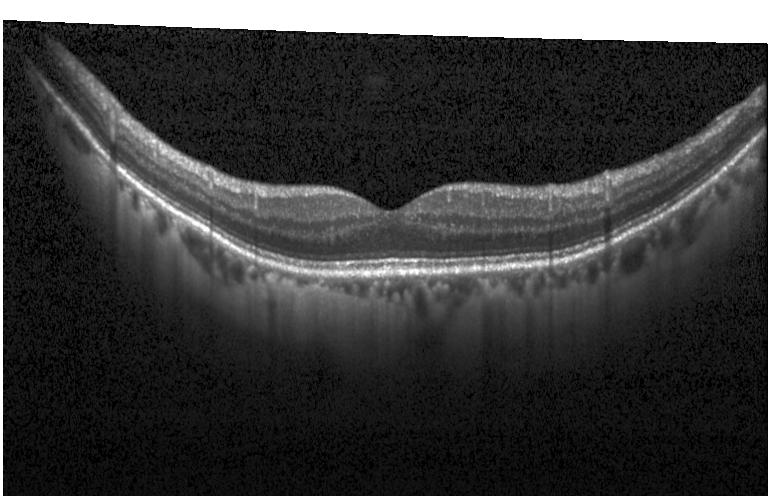
Horizontal scan through the fovea, instrument: Heidelberg Spectralis, spectral-domain OCT, retinal OCT cross-section — Neither choroidal neovascularization, diabetic macular edema, nor drusen.